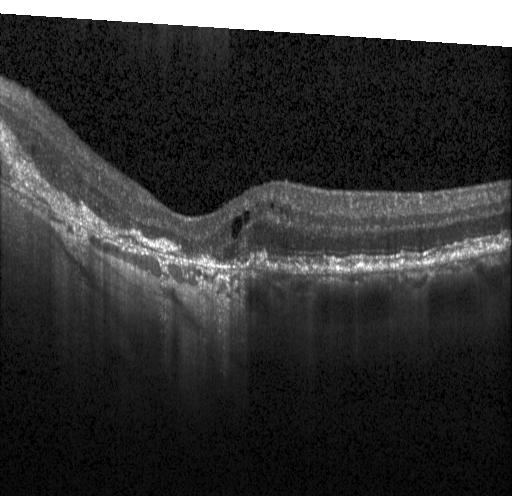

Dx: choroidal neovascularization.